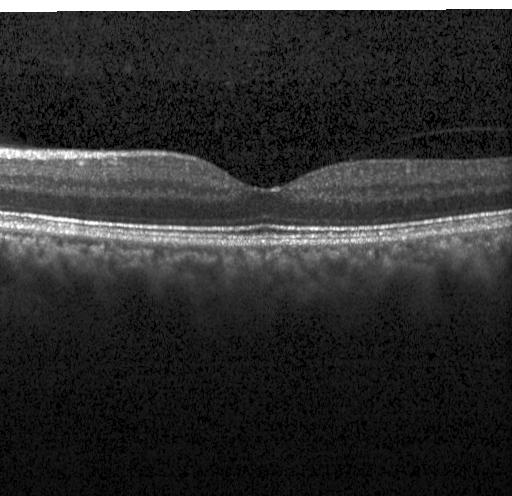
OCT scan showing no choroidal neovascularization, no diabetic macular edema, and no drusen.